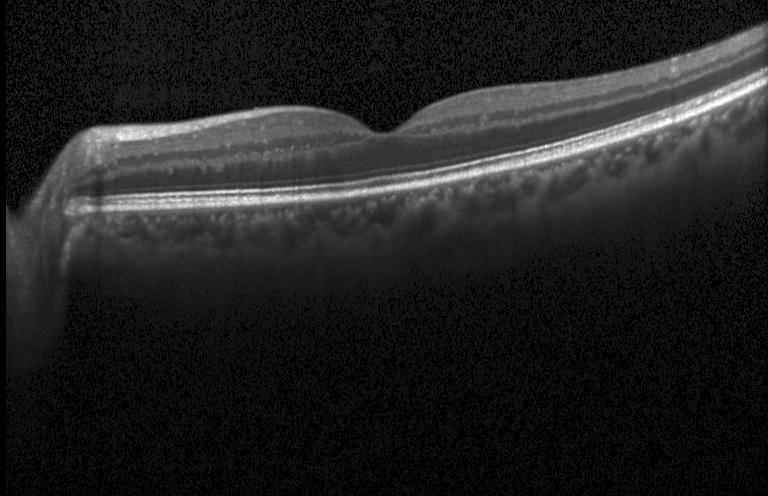
OCT finding: neither choroidal neovascularization, diabetic macular edema, nor drusen.